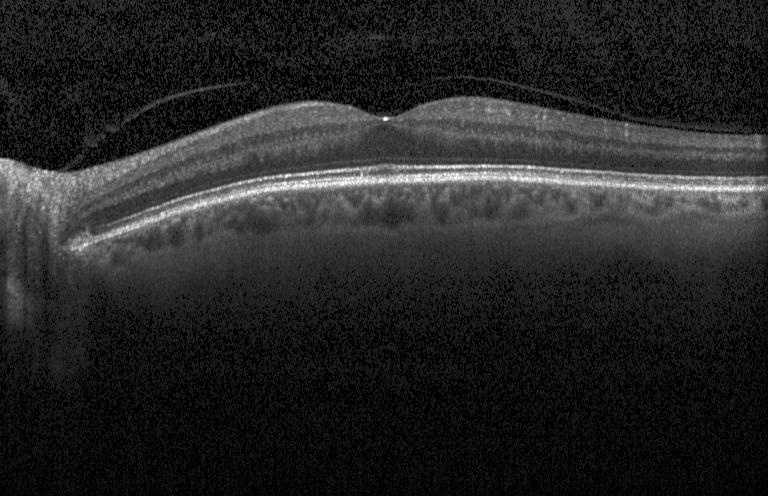

Heidelberg Spectralis · retinal OCT cross-section
Assessment: neither choroidal neovascularization, diabetic macular edema, nor drusen.